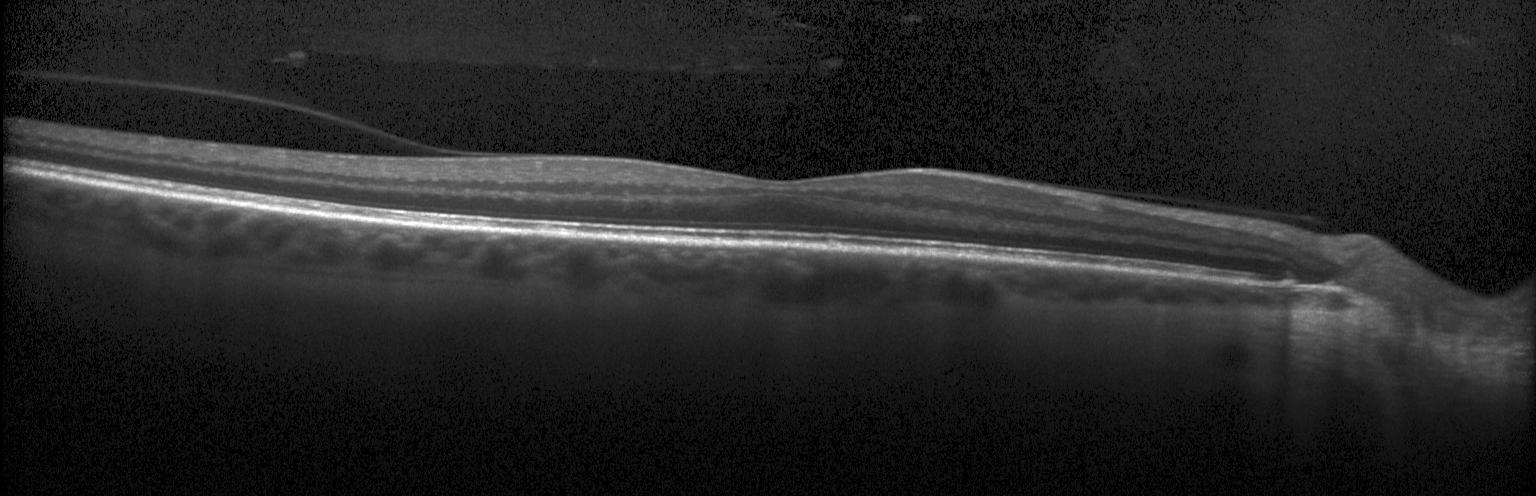

Retinal OCT cross-section · spectral-domain OCT. Impression: no choroidal neovascularization, no diabetic macular edema, and no drusen.